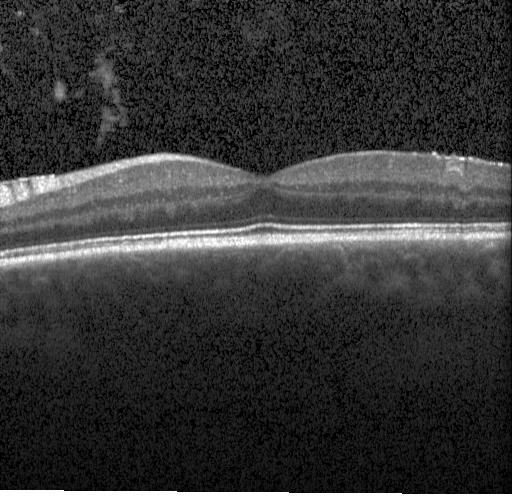
Instrument: Heidelberg Spectralis. OCT B-scan
This B-scan demonstrates neither CNV, DME, nor drusen.